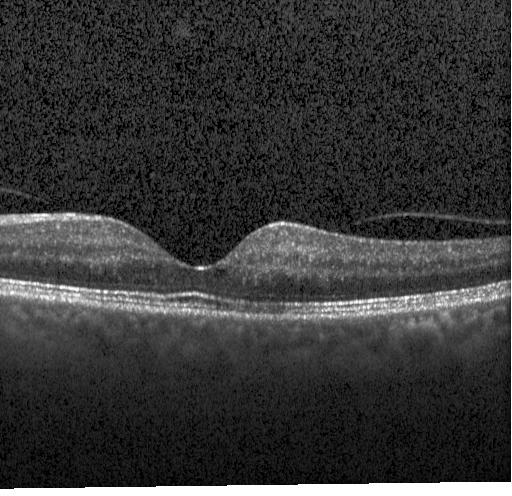
Acquired on a Heidelberg Spectralis. Optical coherence tomography scan.
The scan shows no evidence of choroidal neovascularization, diabetic macular edema, or drusen.